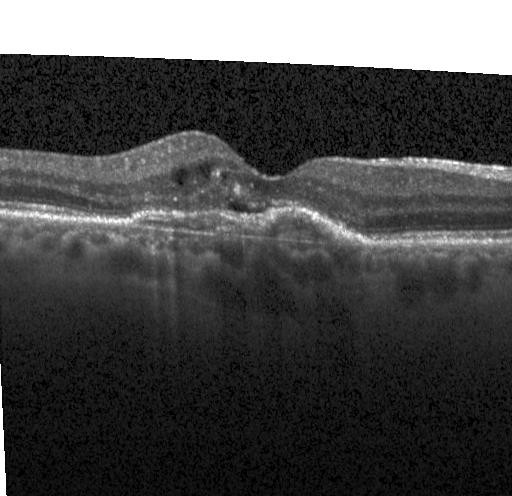
Retinal OCT cross-section. Macular scan — This B-scan demonstrates CNV.